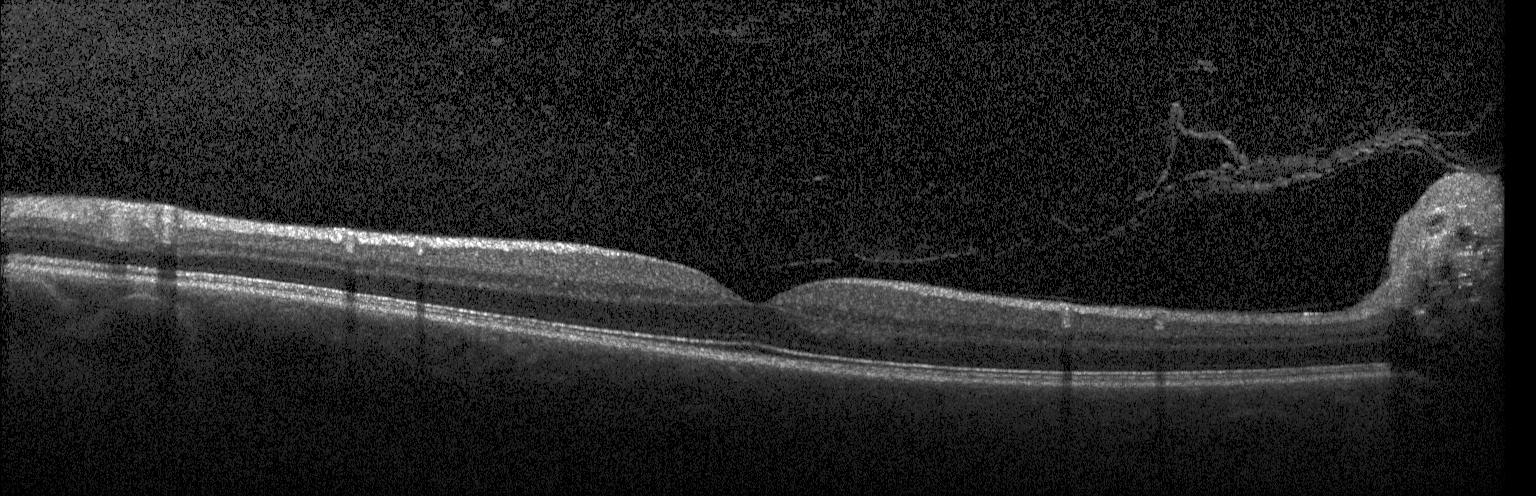
Spectral-domain optical coherence tomography; retinal OCT cross-section; macular scan — Impression: neither choroidal neovascularization, diabetic macular edema, nor drusen.